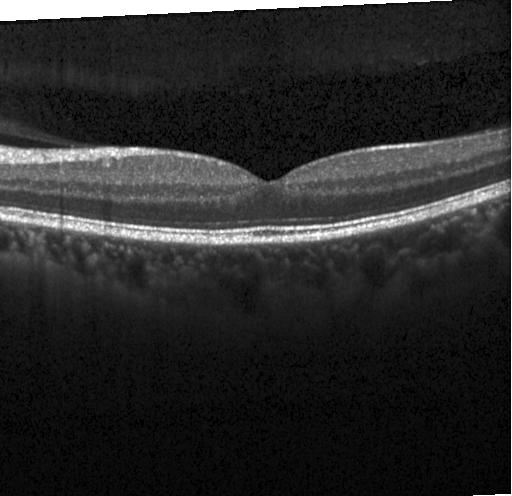
Macular OCT demonstrating no evidence of choroidal neovascularization, diabetic macular edema, or drusen.